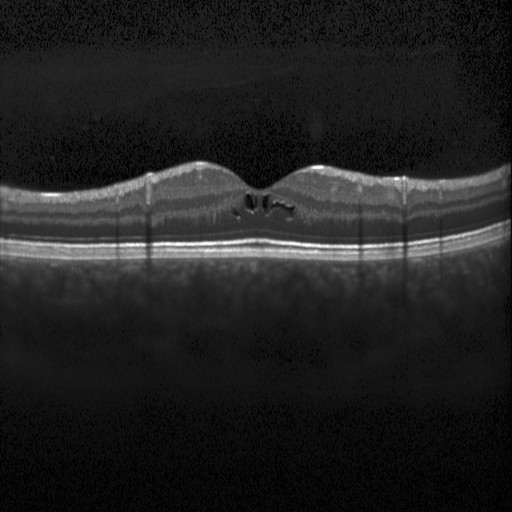 Assessment: diabetic macular edema (DME).